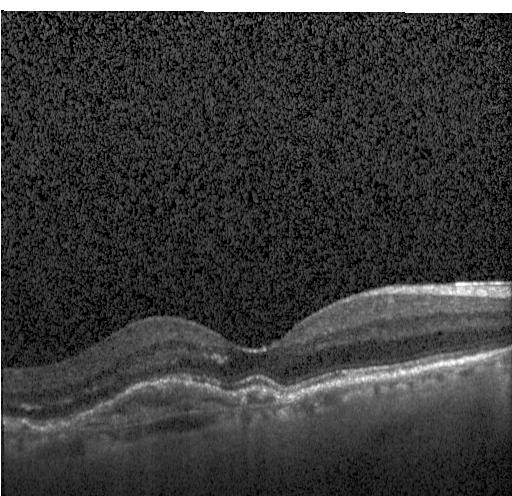
Macular scan, retinal OCT cross-section, Heidelberg Spectralis.
Finding: a choroidal neovascular membrane.